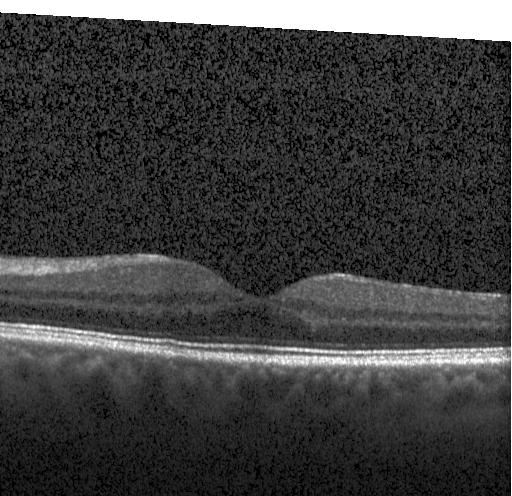

Spectral-domain OCT. Optical coherence tomography scan. Heidelberg Spectralis. Fovea-centered
Diagnosis: no evidence of choroidal neovascularization, diabetic macular edema, or drusen.